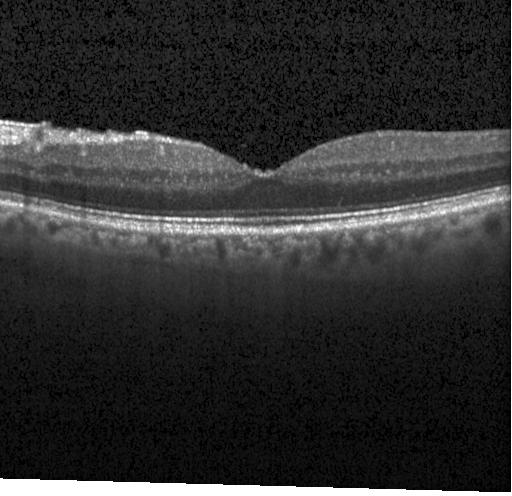

Horizontal scan through the fovea. Retinal OCT B-scan
Diagnosis: no choroidal neovascularization, diabetic macular edema, or drusen.